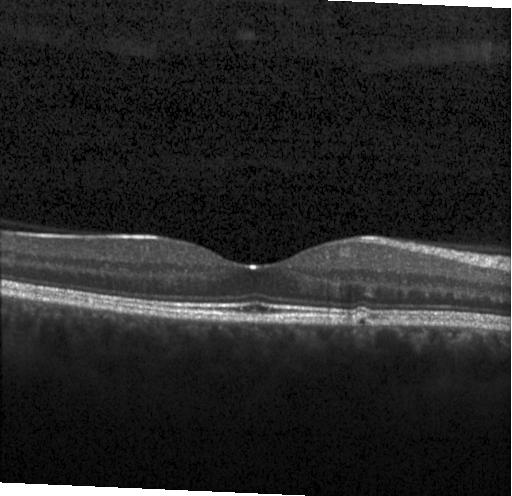

Sub-RPE drusenoid deposits.